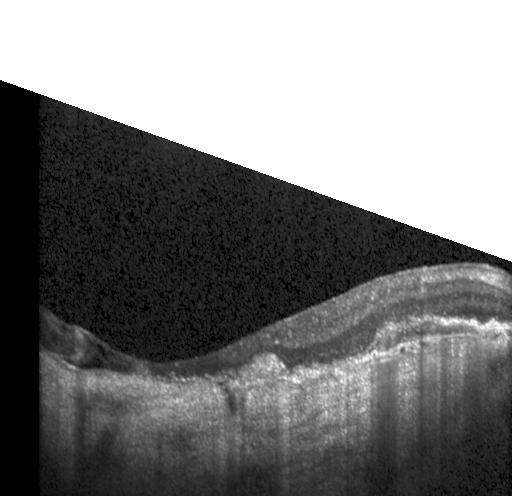 Heidelberg Spectralis; spectral-domain optical coherence tomography; macular scan; optical coherence tomography B-scan. Assessment: CNV.